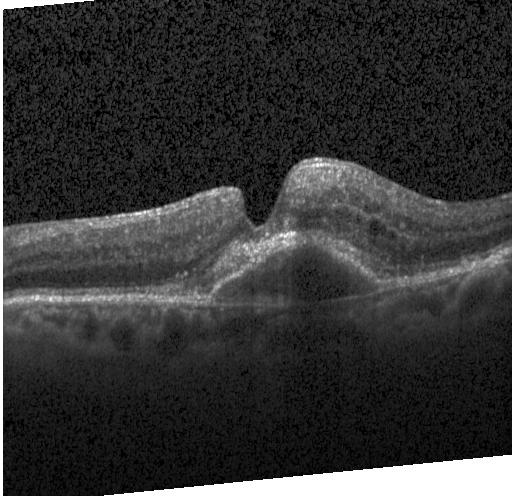

Heidelberg Spectralis. Spectral-domain optical coherence tomography. Retinal OCT B-scan. Horizontal scan through the fovea
The scan shows a choroidal neovascular membrane.